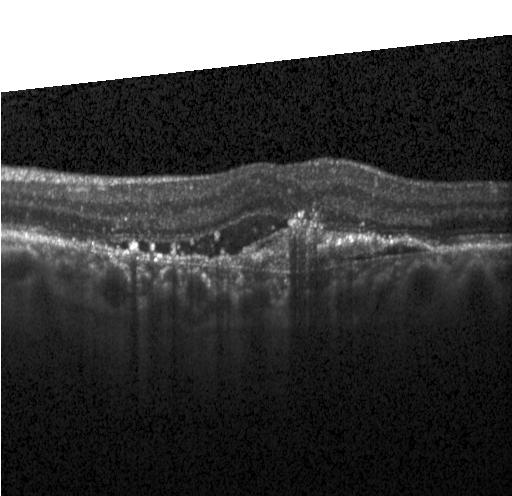

OCT line scan; horizontal scan through the fovea. OCT finding: a choroidal neovascular membrane.